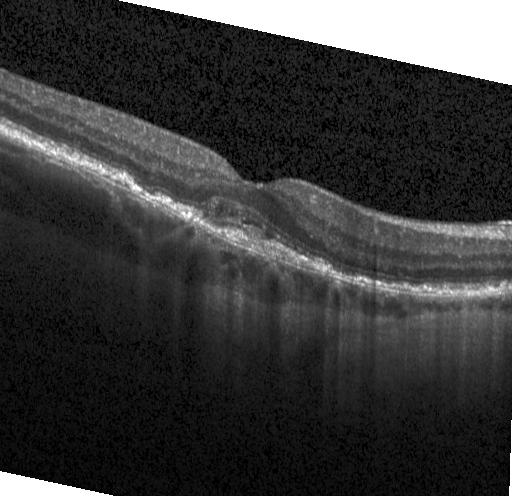
Optical coherence tomography scan · Heidelberg Spectralis · horizontal scan through the fovea — Finding: choroidal neovascularization.